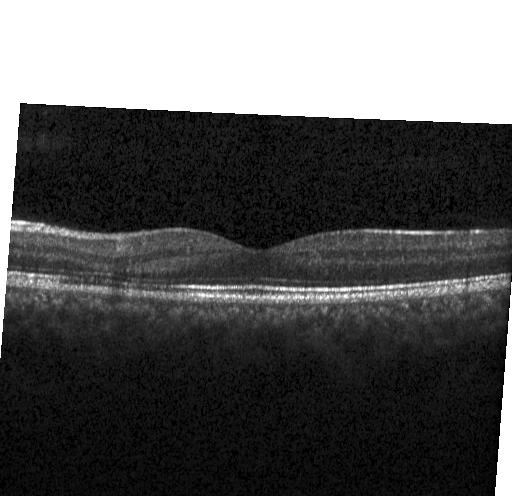

Spectral-domain optical coherence tomography · optical coherence tomography scan · macular scan · Heidelberg Spectralis OCT system. Finding: no choroidal neovascularization, no diabetic macular edema, and no drusen.